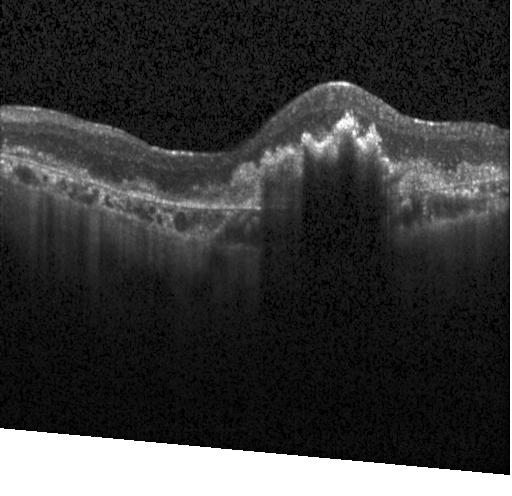

OCT B-scan showing a choroidal neovascular membrane.